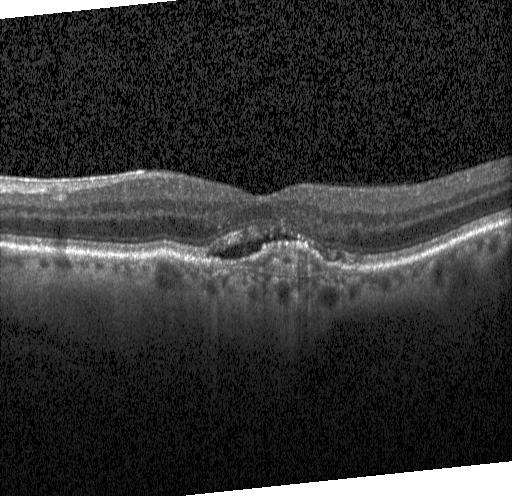

Optical coherence tomography scan; spectral-domain optical coherence tomography; instrument: Heidelberg Spectralis.
Dx: a choroidal neovascular membrane.